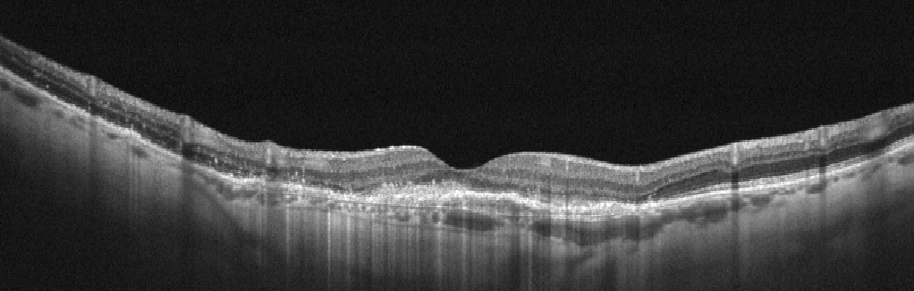 Oculus dexter; OCT line scan.
Finding: age-related macular degeneration (AMD).